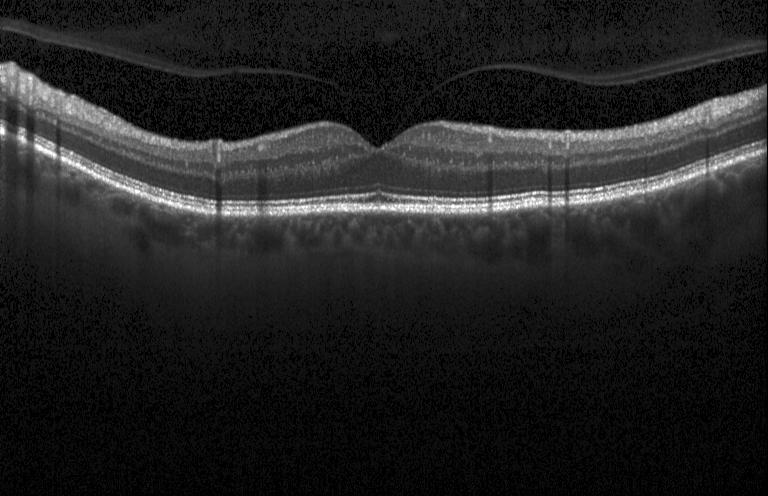

No CNV, no DME, and no drusen.